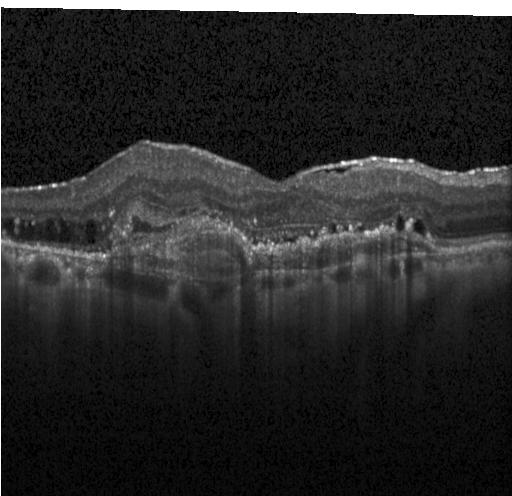
Assessment: a choroidal neovascular membrane.